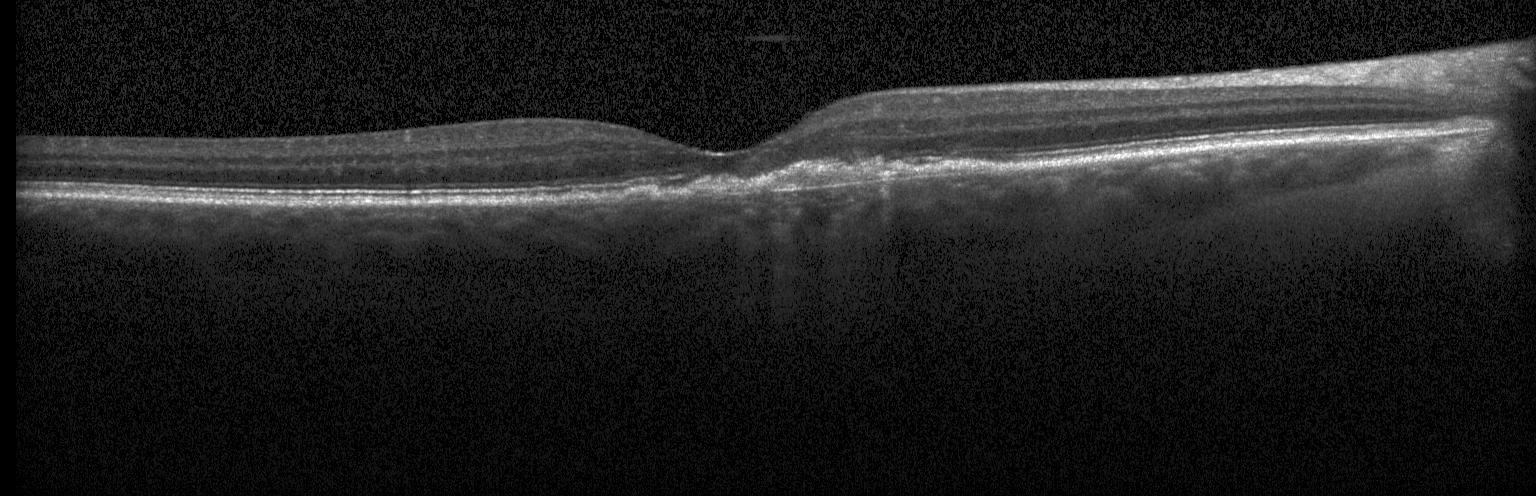
Impression: choroidal neovascularization.